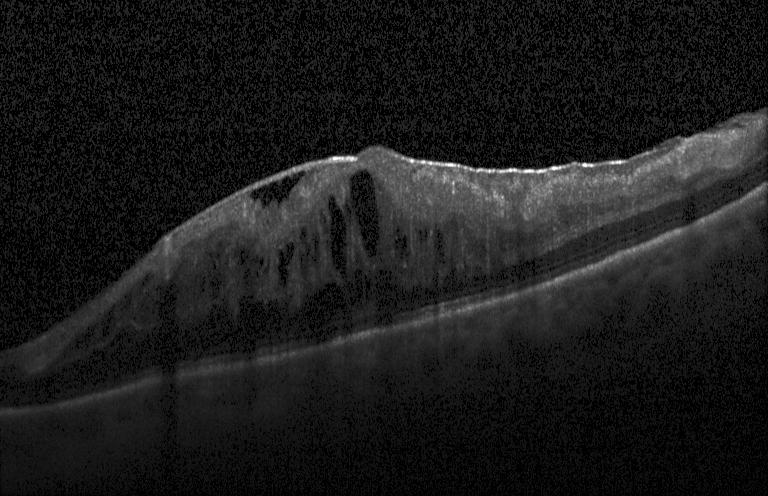

Impression: diabetic macular edema (DME).